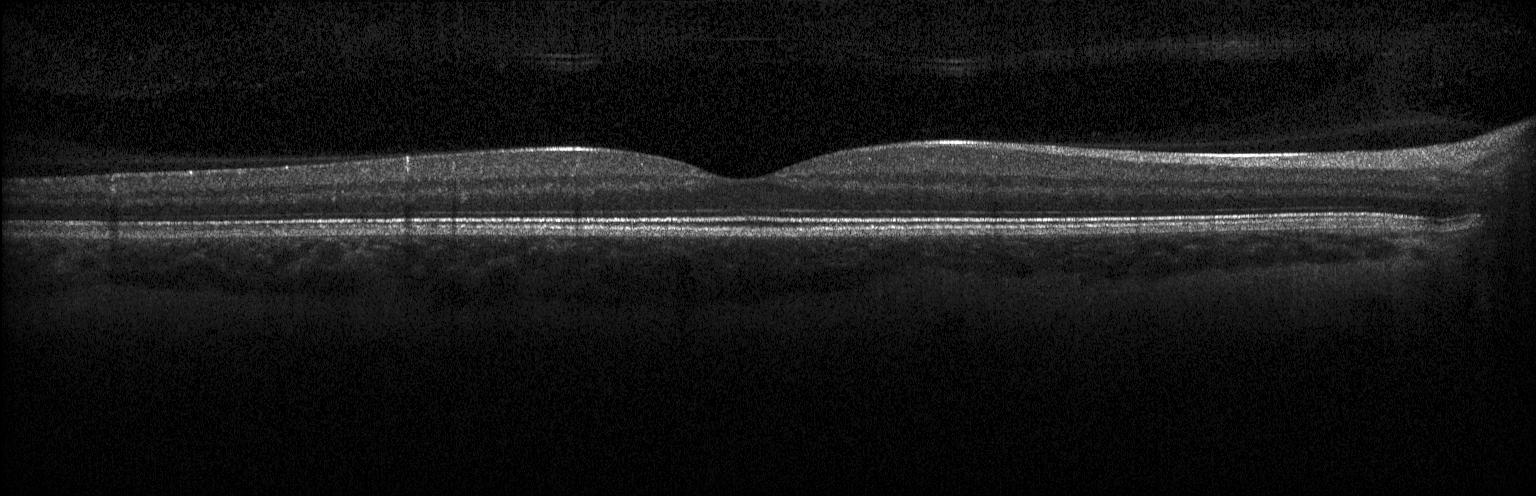

OCT line scan; Heidelberg Spectralis; spectral-domain optical coherence tomography.
Dx: no evidence of choroidal neovascularization, diabetic macular edema, or drusen.